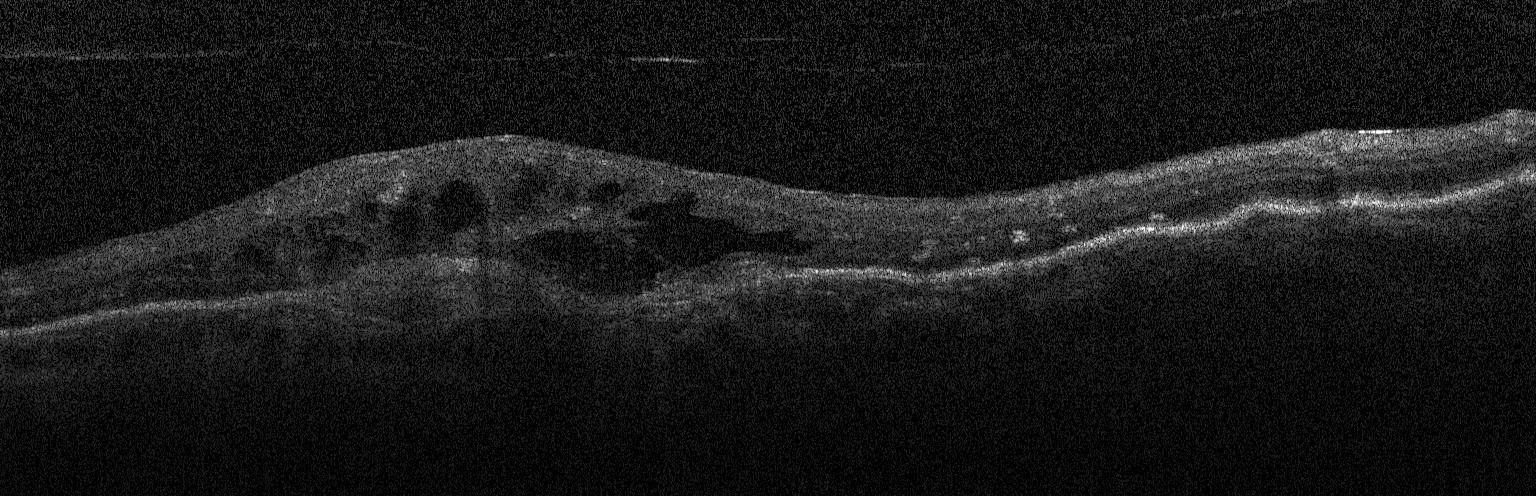
Fovea-centered. OCT B-scan — Finding: CNV.